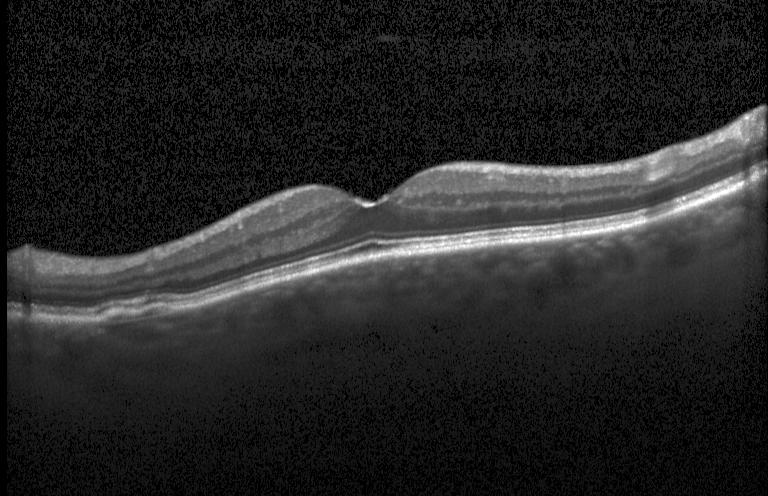
Instrument: Heidelberg Spectralis. Horizontal scan through the fovea. SD-OCT. OCT B-scan — Finding: CNV.